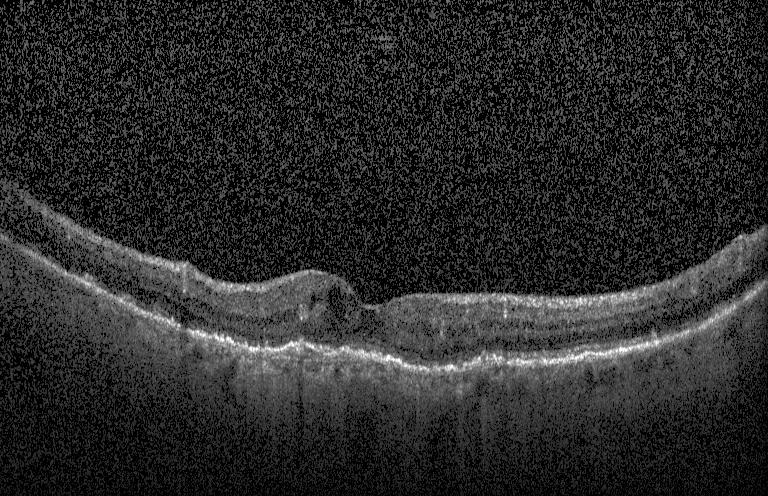

Macular scan · Heidelberg Spectralis OCT system · optical coherence tomography B-scan. The scan shows choroidal neovascularization.